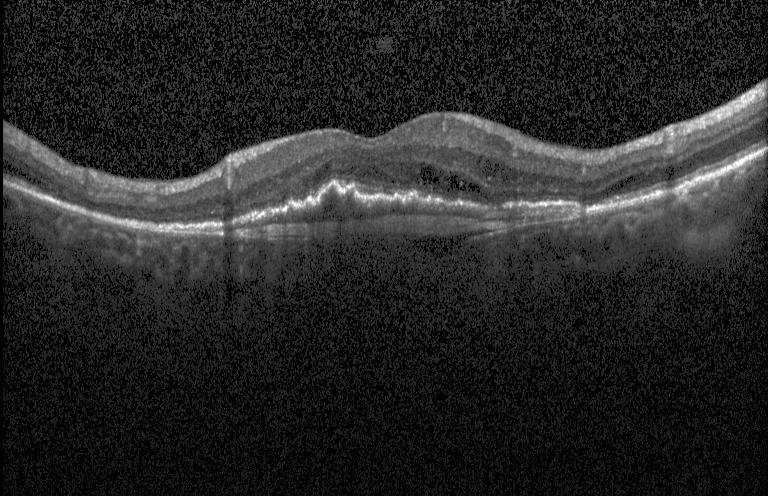 OCT B-scan — Finding: a choroidal neovascular membrane.